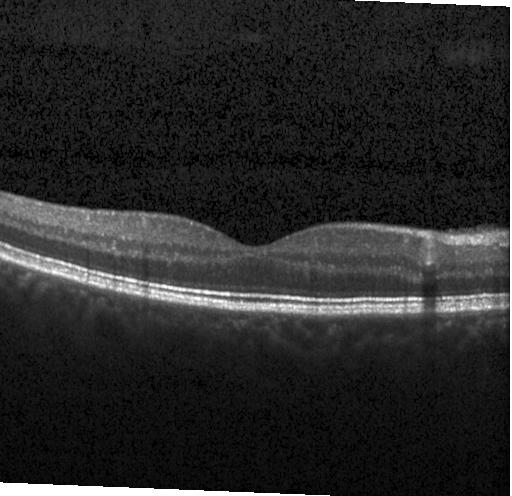 Optical coherence tomography B-scan. Horizontal scan through the fovea. Acquired on a Heidelberg Spectralis
Diagnosis: no evidence of choroidal neovascularization, diabetic macular edema, or drusen.